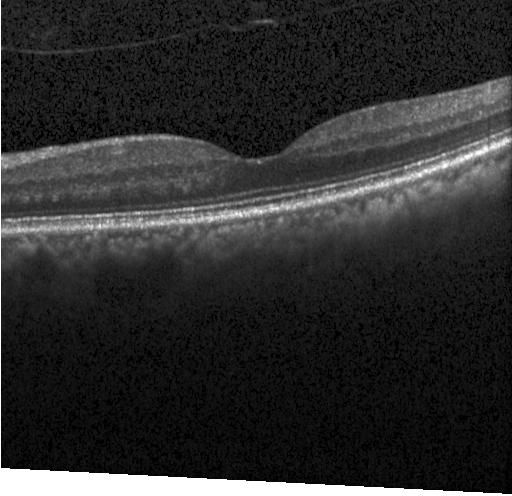
OCT line scan. SD-OCT. Centered on the fovea. Instrument: Heidelberg Spectralis — Finding: no CNV, no DME, and no drusen.